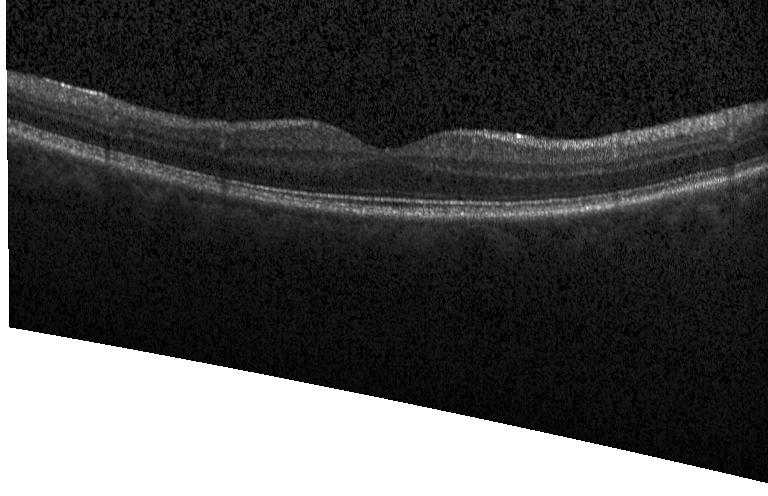 Heidelberg Spectralis OCT system; horizontal scan through the fovea; OCT B-scan; spectral-domain OCT.
Impression: neither choroidal neovascularization, diabetic macular edema, nor drusen.